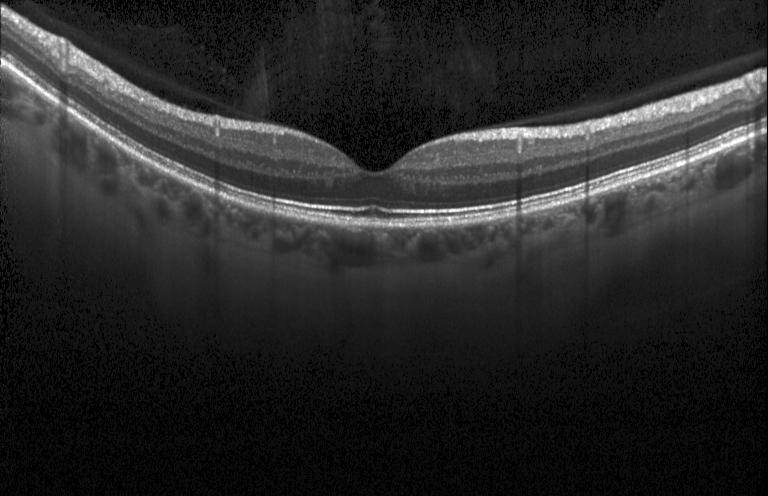

Heidelberg Spectralis OCT system; OCT B-scan.
Impression: no evidence of choroidal neovascularization, diabetic macular edema, or drusen.